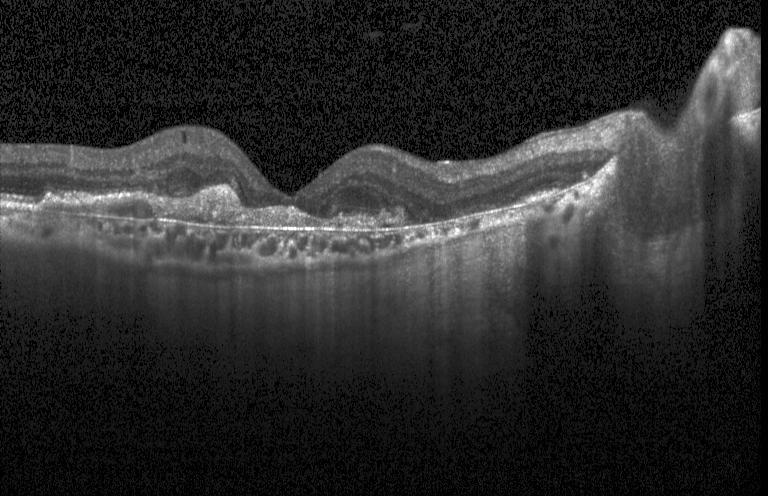 Optical coherence tomography B-scan. Centered on the fovea. Spectral-domain optical coherence tomography. Instrument: Heidelberg Spectralis.
Impression: a choroidal neovascular membrane.